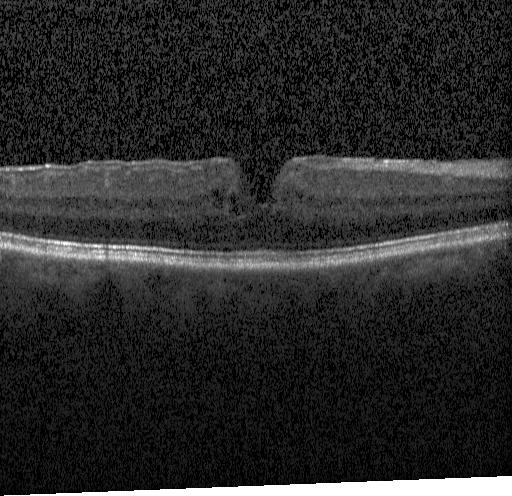

Impression: DME.